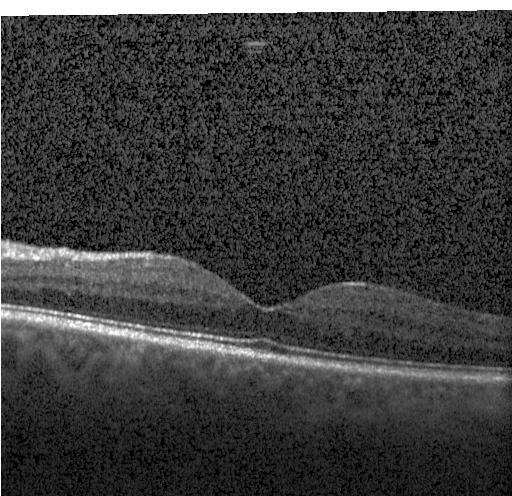

Optical coherence tomography B-scan; fovea-centered; Heidelberg Spectralis. Diagnosis: no choroidal neovascularization, no diabetic macular edema, and no drusen.